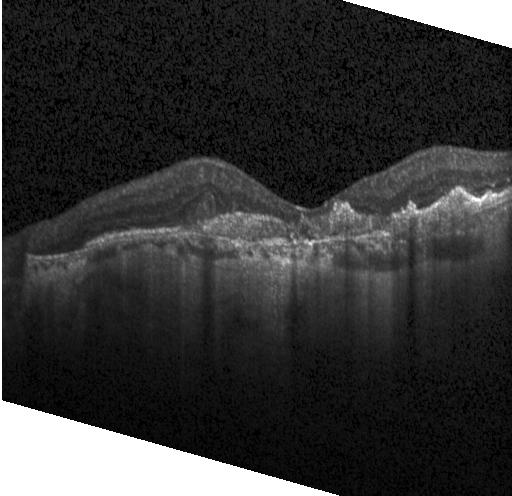 The scan shows choroidal neovascularization (CNV).